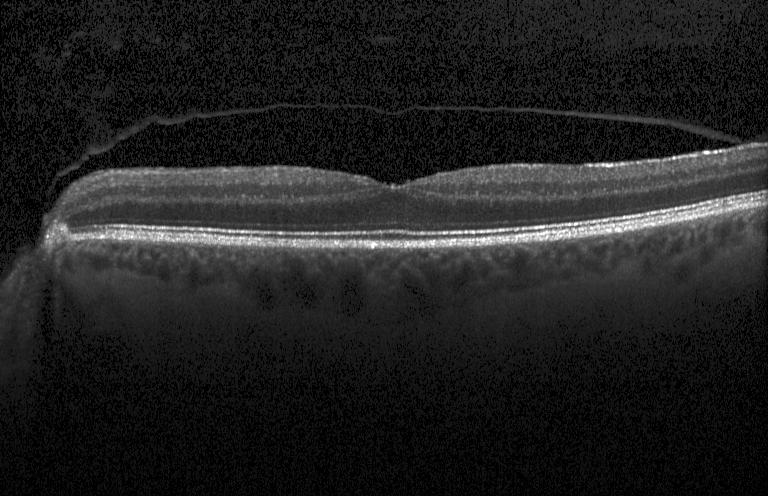 Spectral-domain optical coherence tomography, acquired on a Heidelberg Spectralis, OCT line scan. Impression: neither CNV, DME, nor drusen.